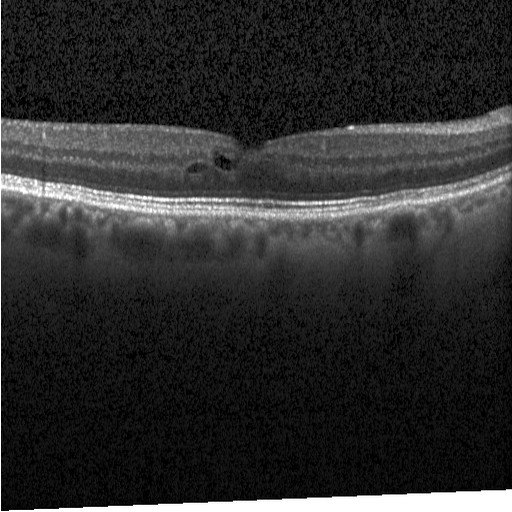
Centered on the fovea · OCT line scan — Diagnosis: DME.